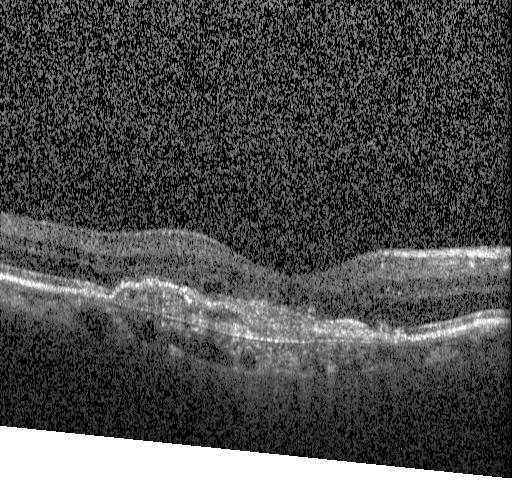
Retinal OCT B-scan. The scan shows a choroidal neovascular membrane.